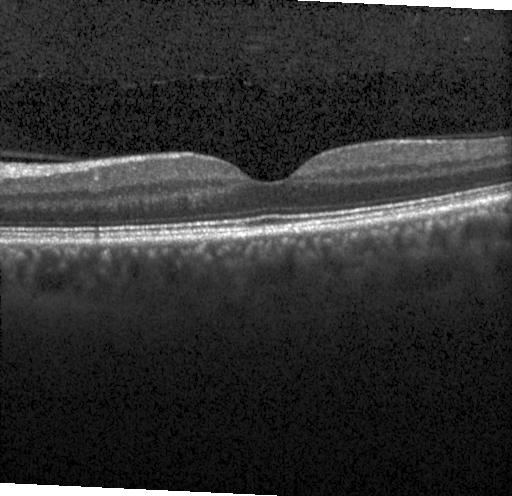 Retinal OCT cross-section showing neither choroidal neovascularization, diabetic macular edema, nor drusen.